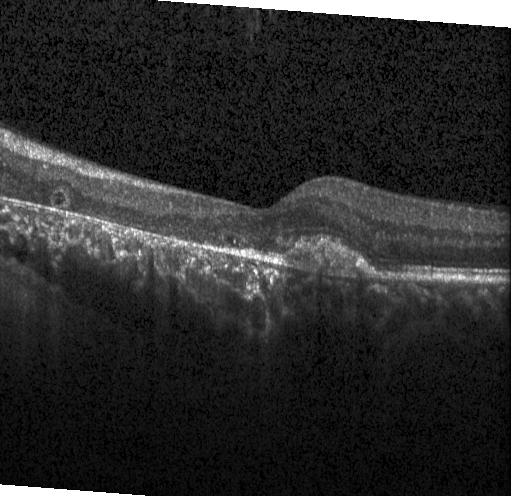

Finding: a choroidal neovascular membrane.